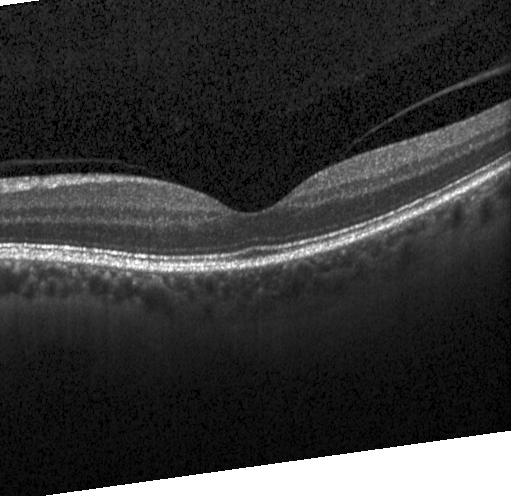
Diagnosis: neither CNV, DME, nor drusen.